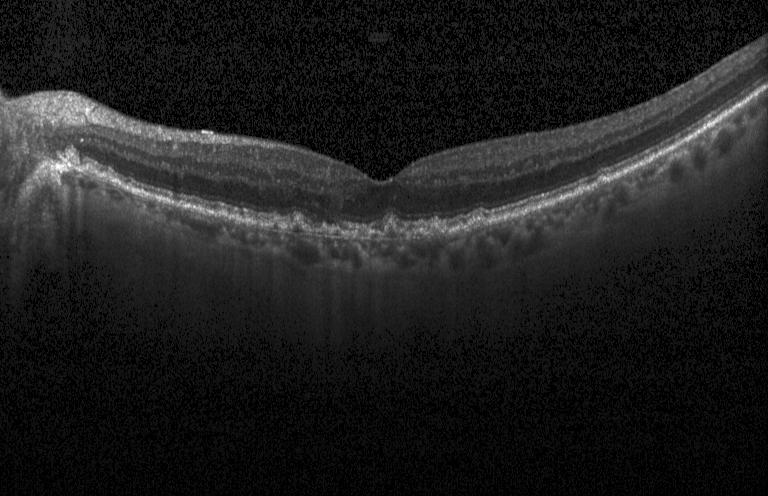
OCT line scan — Impression: multiple drusen.